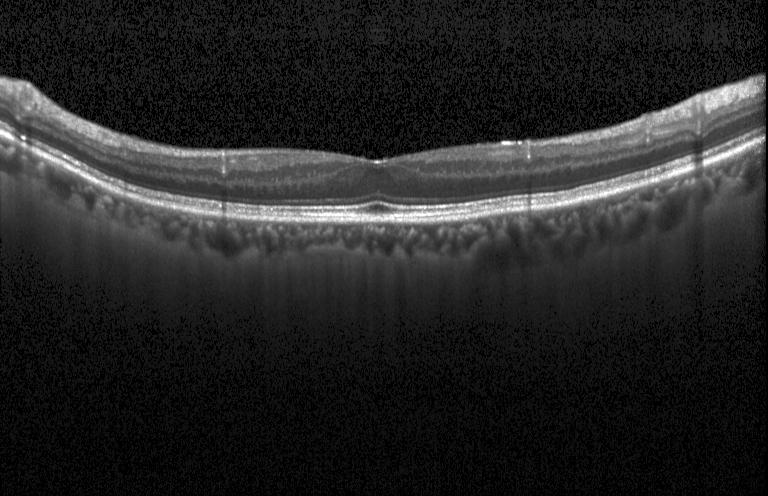
Spectral-domain OCT B-scan: no choroidal neovascularization, diabetic macular edema, or drusen.